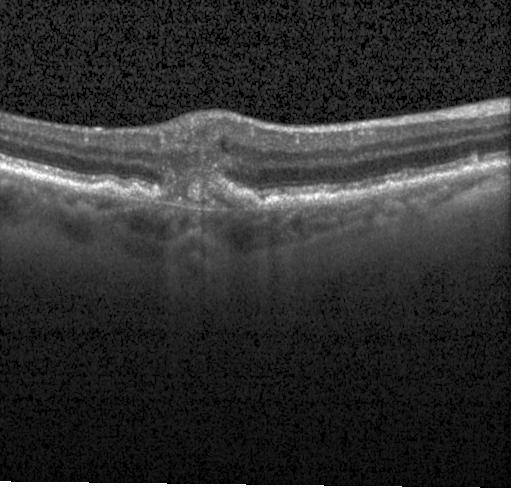 The scan shows choroidal neovascularization (CNV).